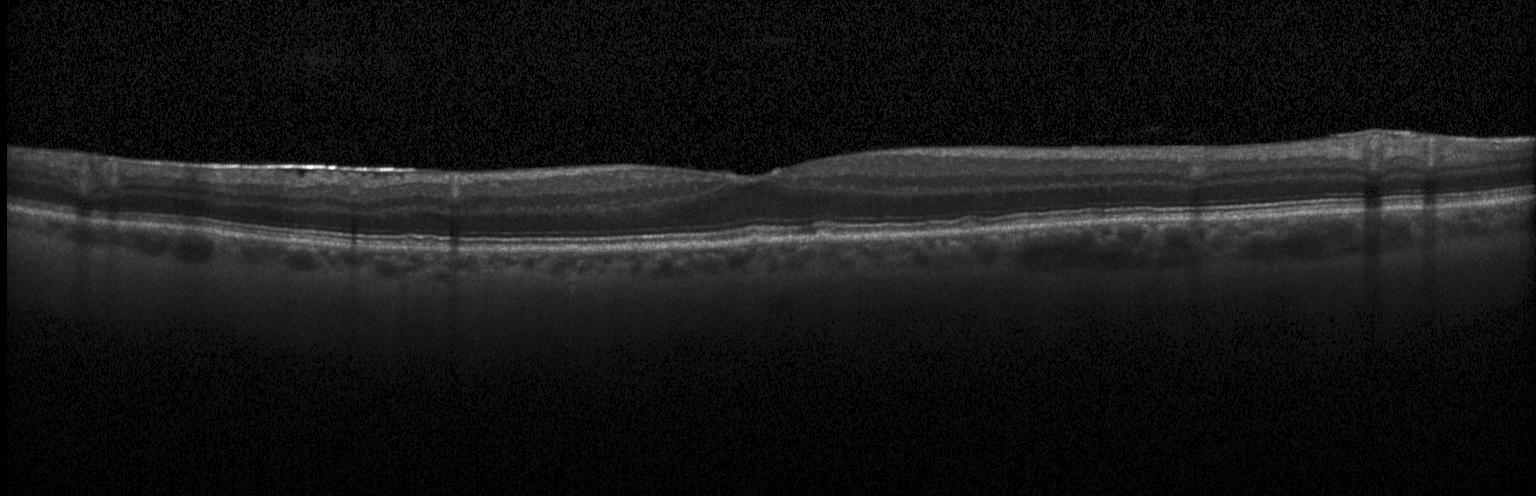 SD-OCT. Retinal OCT cross-section — This B-scan demonstrates sub-RPE drusenoid deposits.